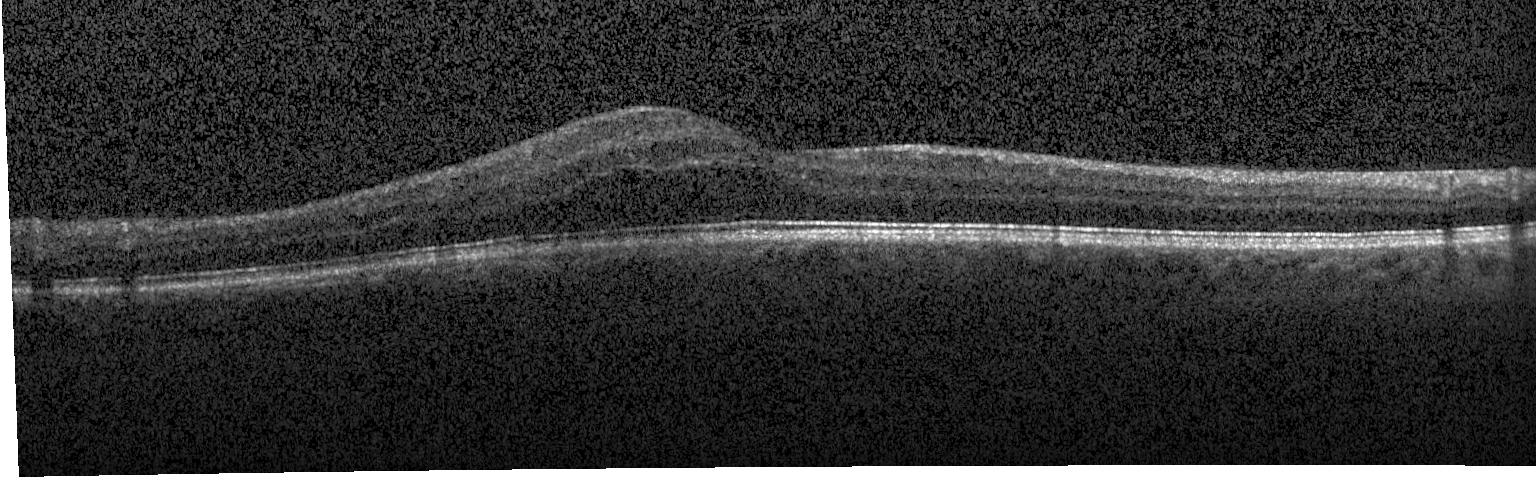 Centered on the fovea. Retinal OCT B-scan. Heidelberg Spectralis OCT system. Spectral-domain OCT — Impression: diabetic macular edema.